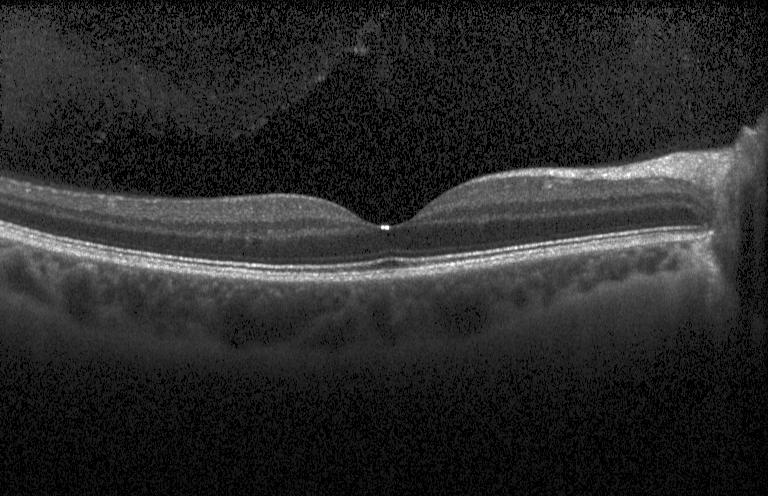 OCT B-scan showing neither choroidal neovascularization, diabetic macular edema, nor drusen.